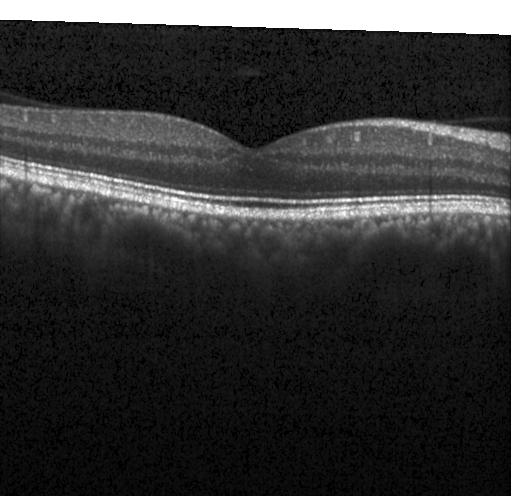
OCT finding: no choroidal neovascularization, no diabetic macular edema, and no drusen.